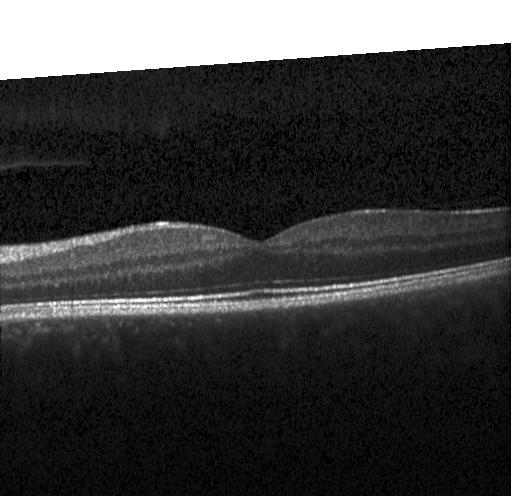 OCT B-scan; acquired on a Heidelberg Spectralis; macular scan.
Dx: no choroidal neovascularization, no diabetic macular edema, and no drusen.